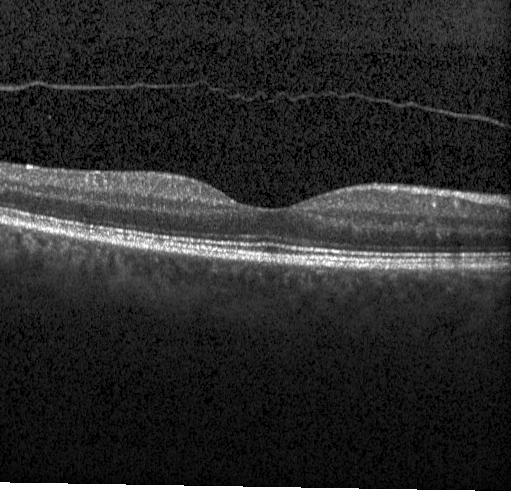 Spectral-domain OCT B-scan: no CNV, DME, or drusen.